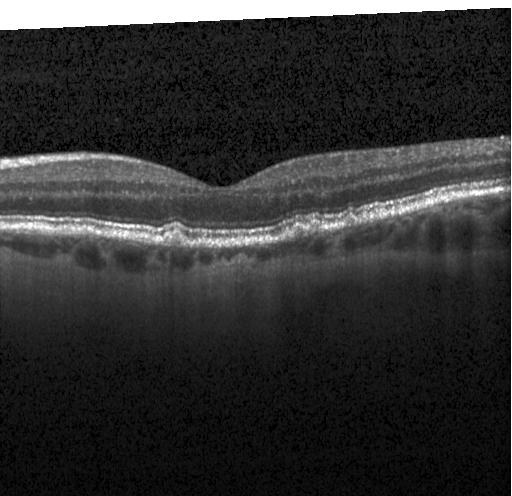

Spectral-domain OCT · retinal OCT B-scan · fovea-centered · acquired on a Heidelberg Spectralis. Finding: multiple drusen.